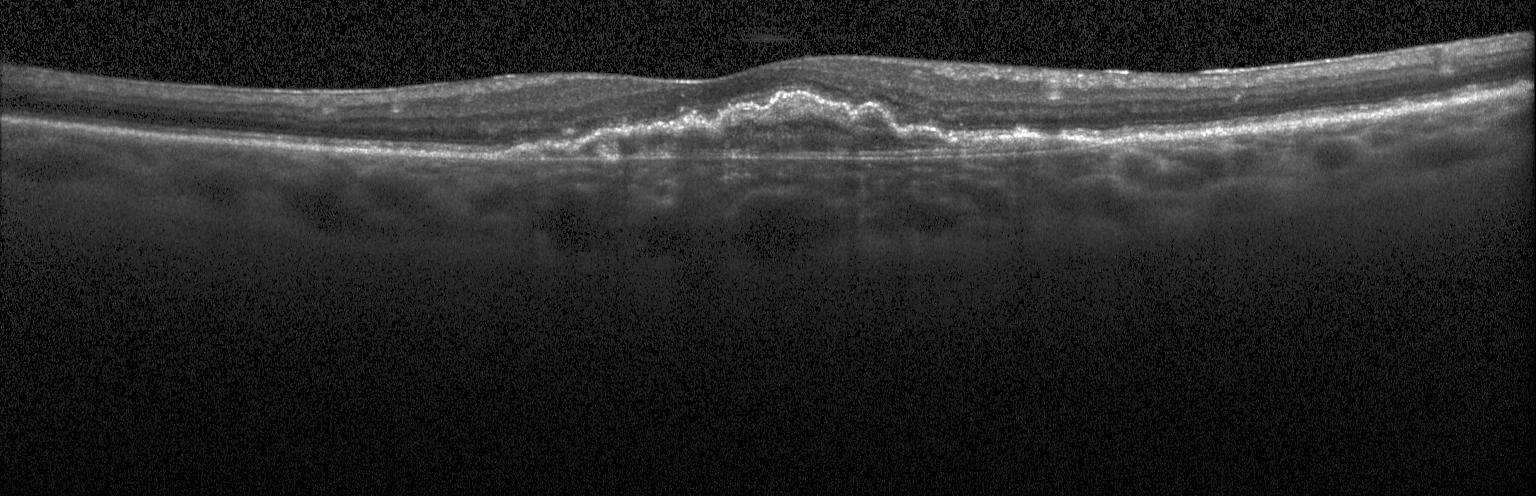 OCT B-scan showing choroidal neovascularization (CNV).